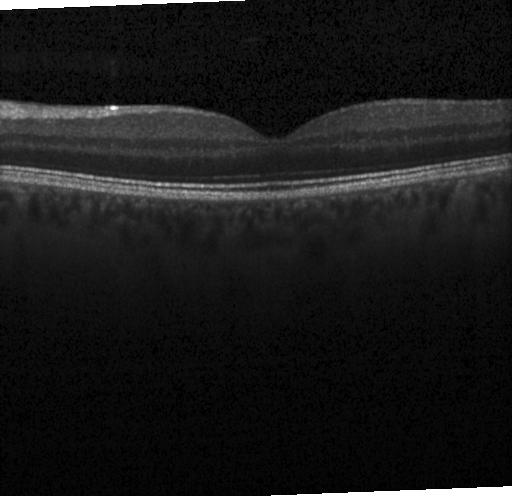

Macular OCT demonstrating no evidence of choroidal neovascularization, diabetic macular edema, or drusen.